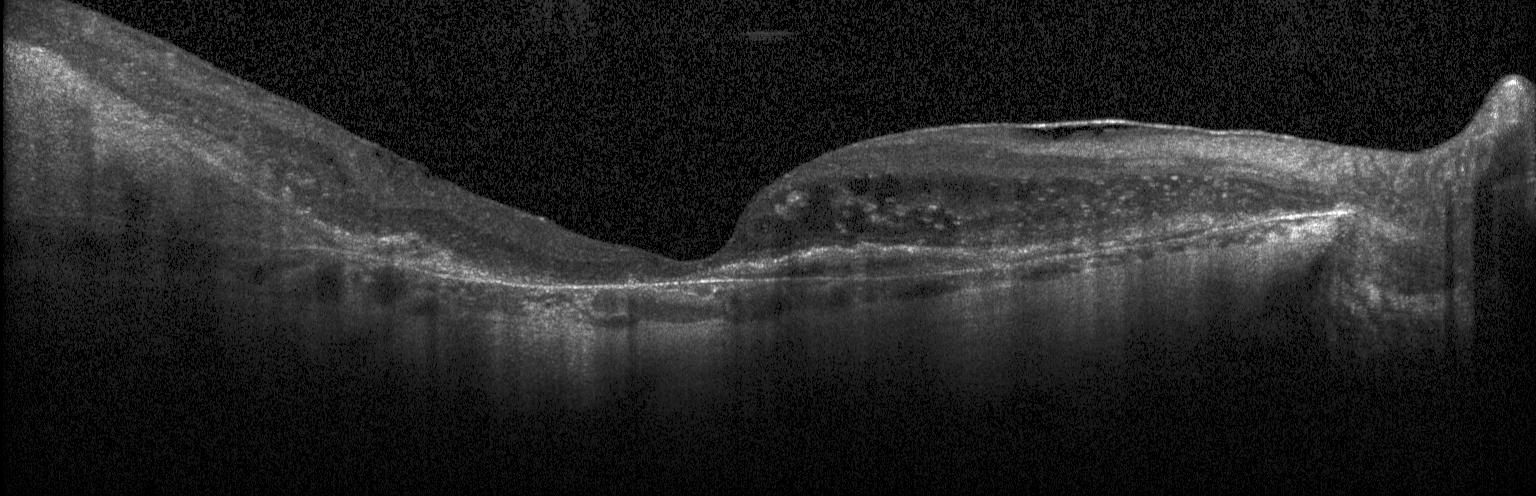

OCT line scan, fovea-centered, instrument: Heidelberg Spectralis, spectral-domain optical coherence tomography. Finding: CNV.